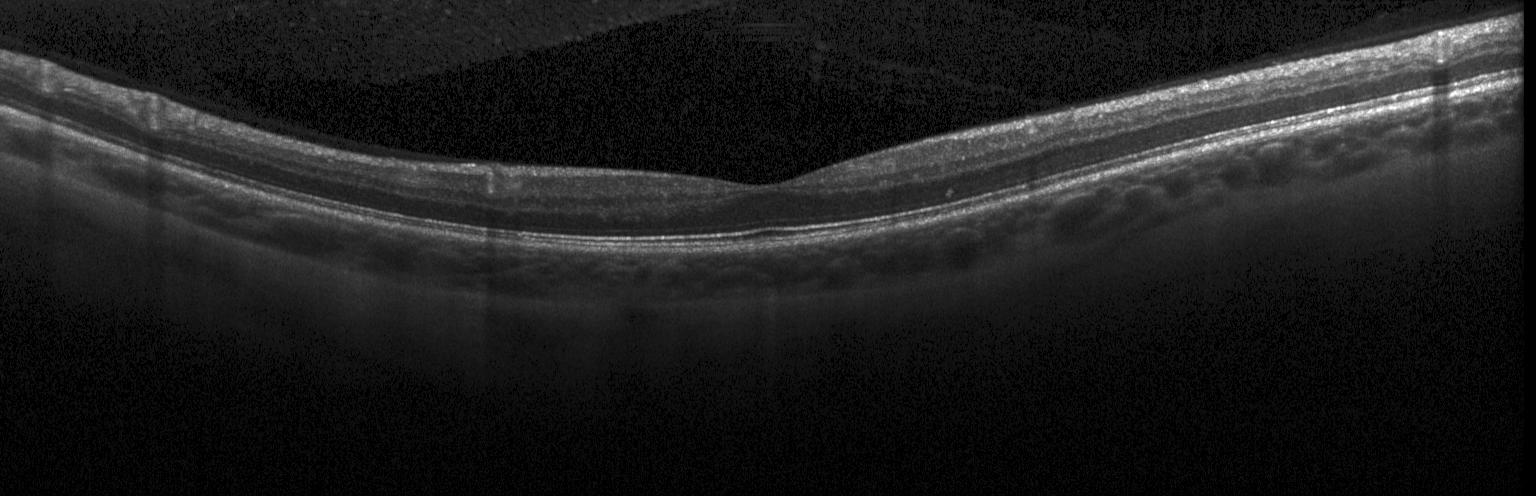

Spectral-domain optical coherence tomography, macular scan, optical coherence tomography B-scan. Finding: no choroidal neovascularization, diabetic macular edema, or drusen.